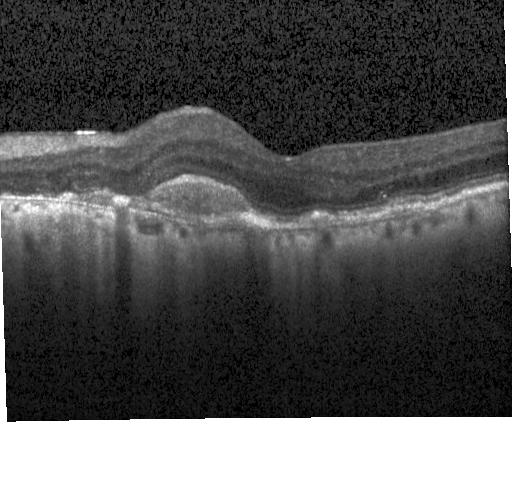
Assessment: choroidal neovascularization.